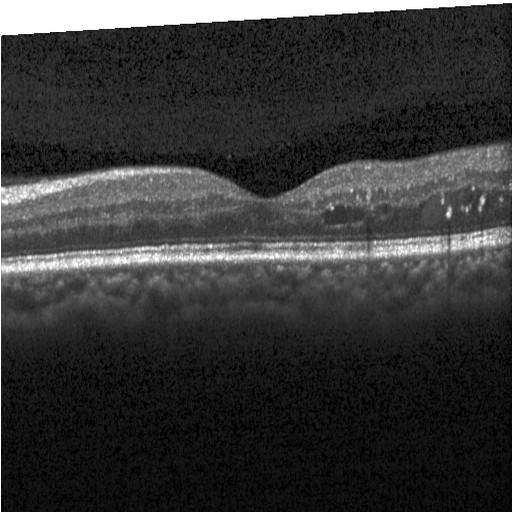 OCT B-scan; centered on the fovea. Diagnosis: diabetic macular edema.